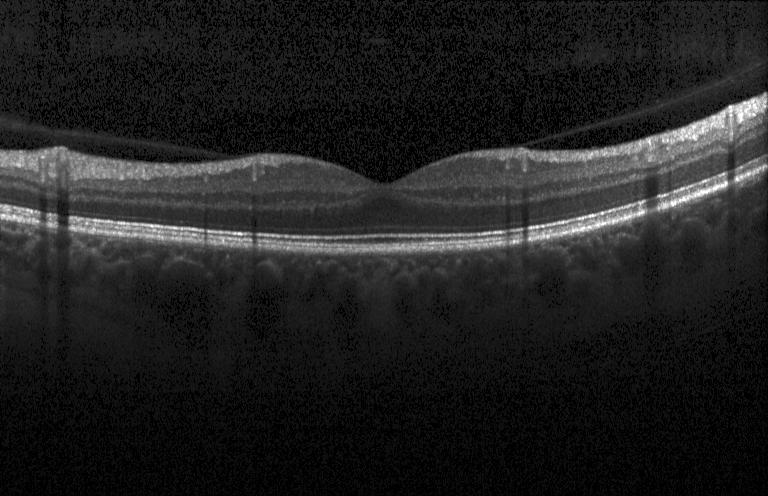
Heidelberg Spectralis; retinal OCT B-scan; centered on the fovea — Macular OCT: no CNV, DME, or drusen.